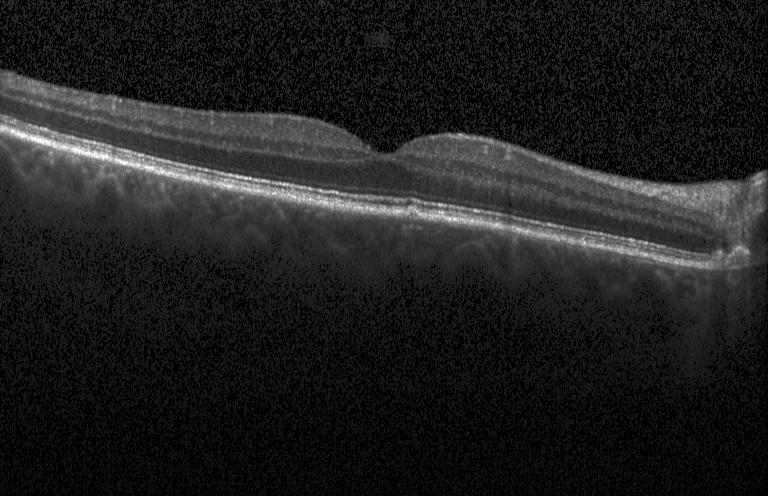
Assessment: sub-RPE drusenoid deposits.